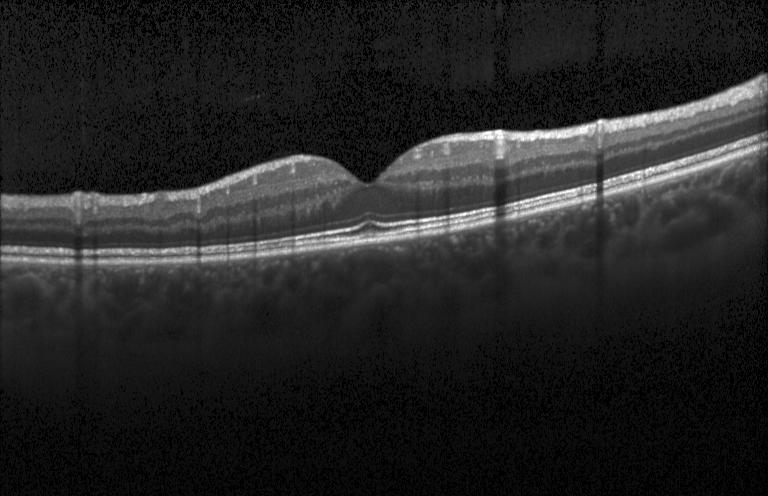 Instrument: Heidelberg Spectralis · optical coherence tomography scan · SD-OCT — Impression: no choroidal neovascularization, no diabetic macular edema, and no drusen.